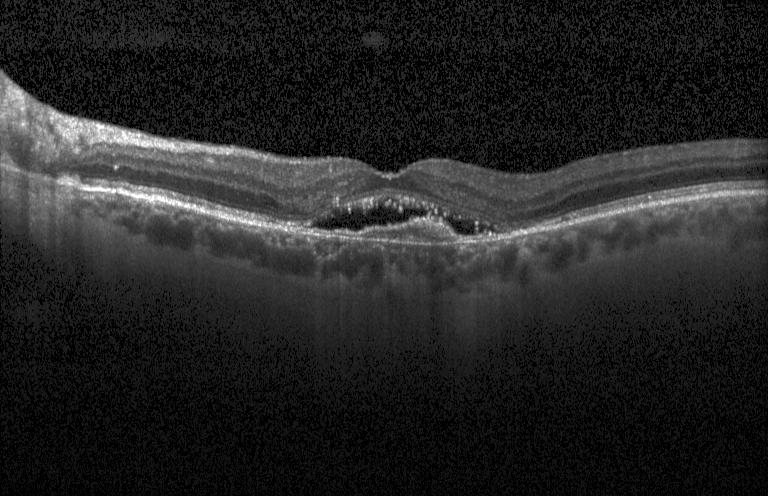
OCT B-scan showing CNV.